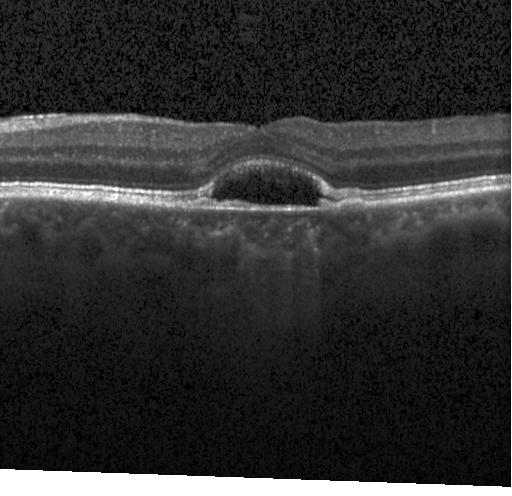
Retinal OCT cross-section showing a choroidal neovascular membrane.